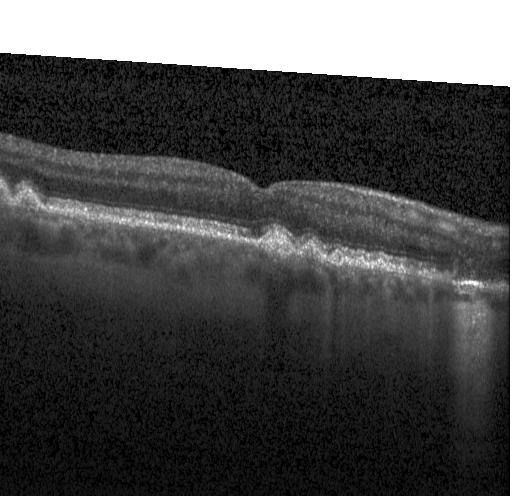

OCT B-scan · Heidelberg Spectralis OCT system · fovea-centered · spectral-domain optical coherence tomography. Impression: drusen.